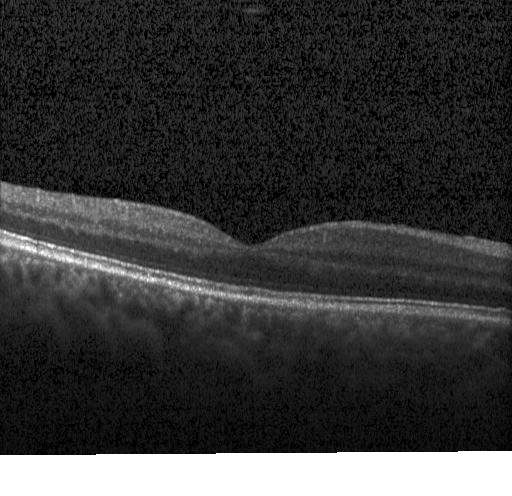

OCT line scan.
Impression: no evidence of choroidal neovascularization, diabetic macular edema, or drusen.